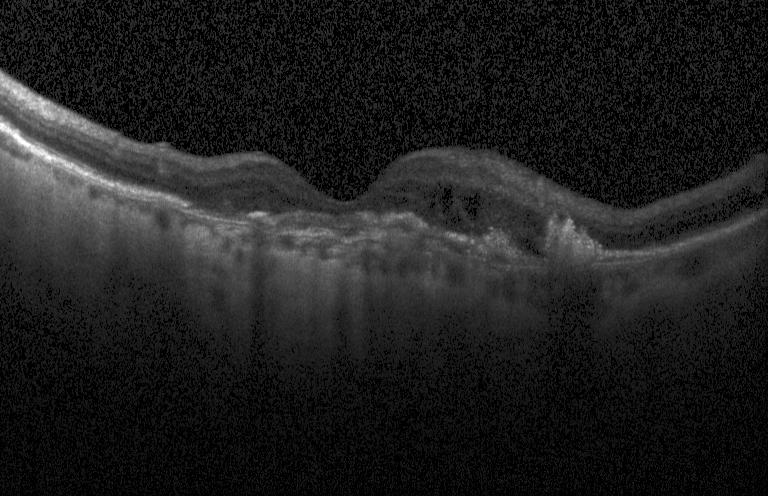

OCT B-scan
The scan shows choroidal neovascularization.